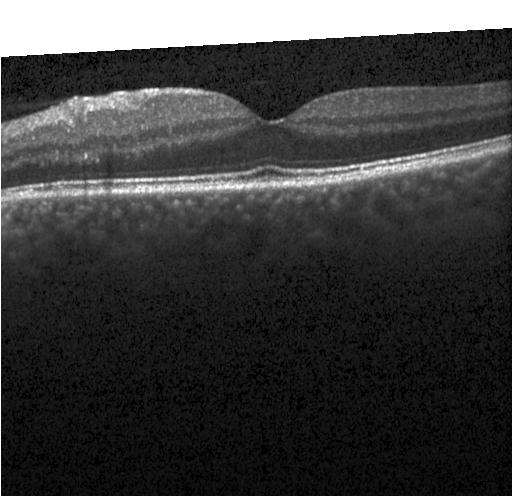 Horizontal scan through the fovea, Heidelberg Spectralis, retinal OCT cross-section.
Assessment: neither CNV, DME, nor drusen.